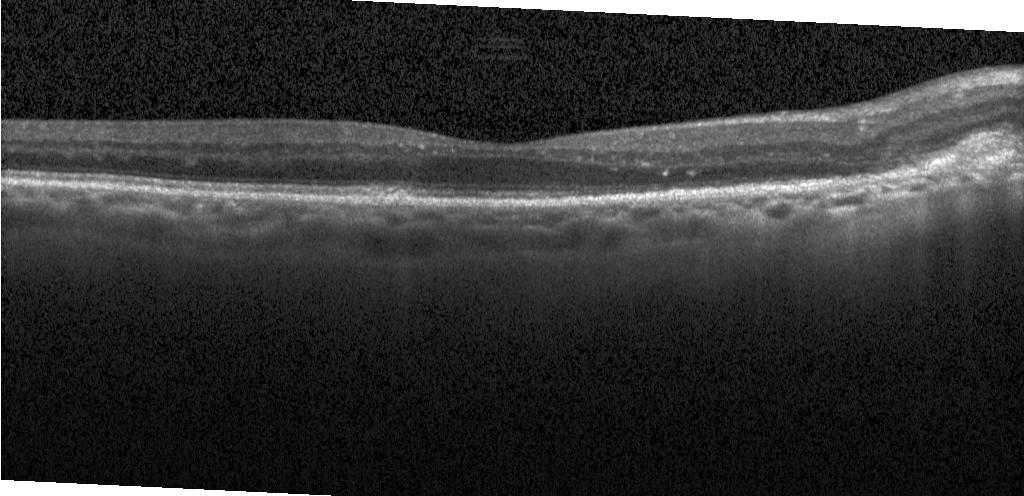
A choroidal neovascular membrane.